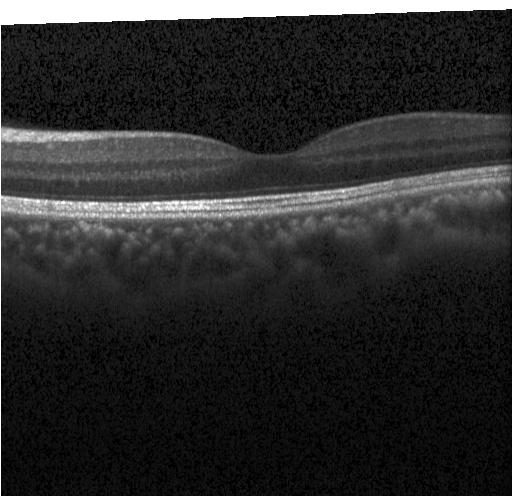 Impression: no choroidal neovascularization, diabetic macular edema, or drusen.